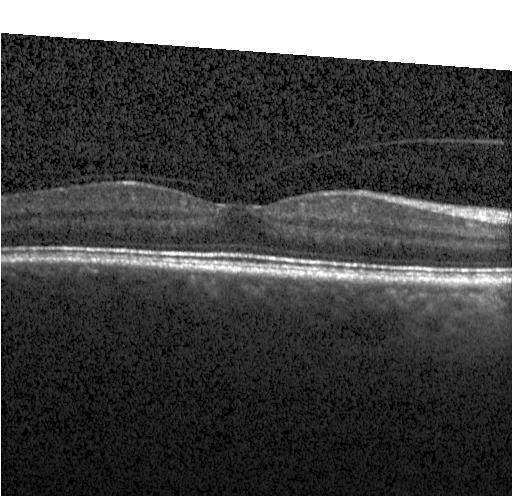 Optical coherence tomography scan — This B-scan demonstrates no CNV, DME, or drusen.